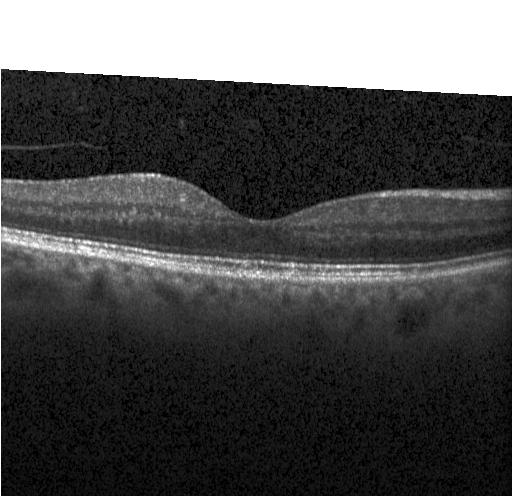
Through the macula, instrument: Heidelberg Spectralis, OCT B-scan, spectral-domain OCT
Finding: no evidence of choroidal neovascularization, diabetic macular edema, or drusen.